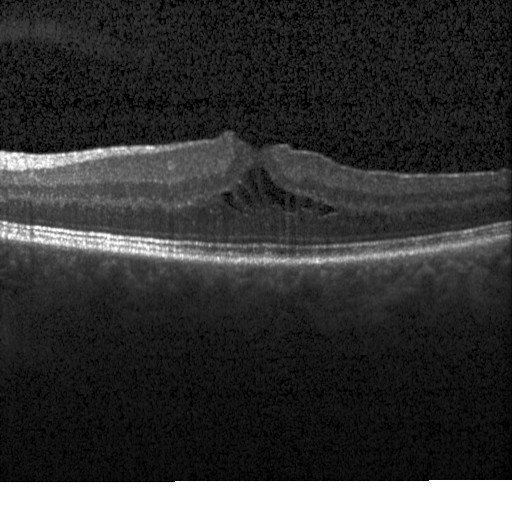 Retinal OCT B-scan.
Impression: diabetic macular edema.